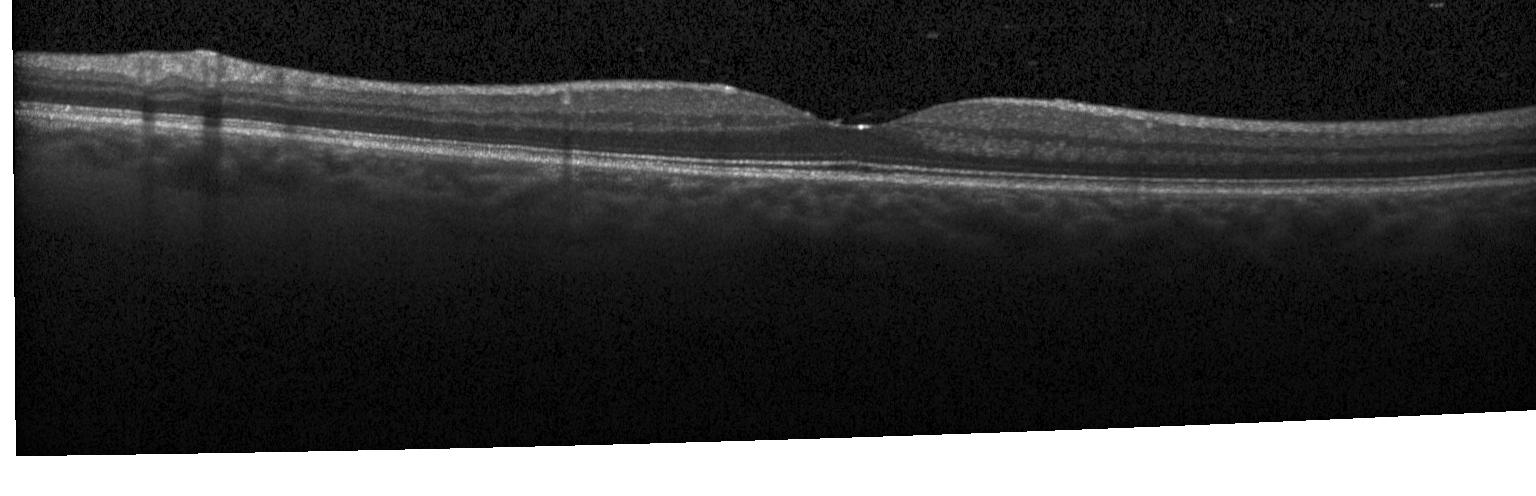 Retinal OCT B-scan, centered on the fovea, instrument: Heidelberg Spectralis, spectral-domain OCT.
Finding: neither choroidal neovascularization, diabetic macular edema, nor drusen.